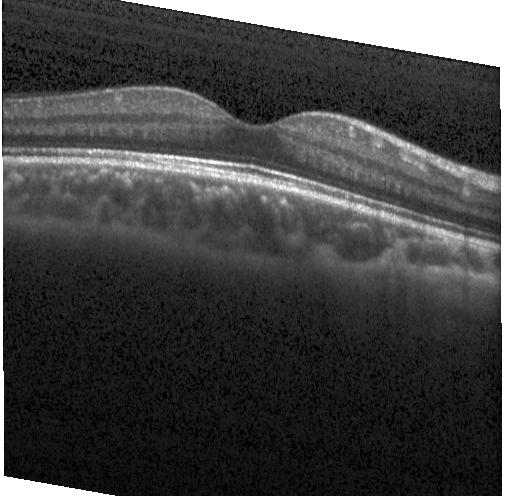 Impression: no choroidal neovascularization, diabetic macular edema, or drusen.